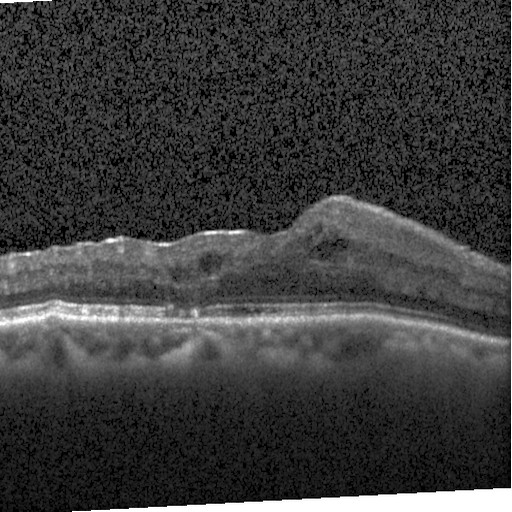 Optical coherence tomography scan — Assessment: diabetic macular edema.